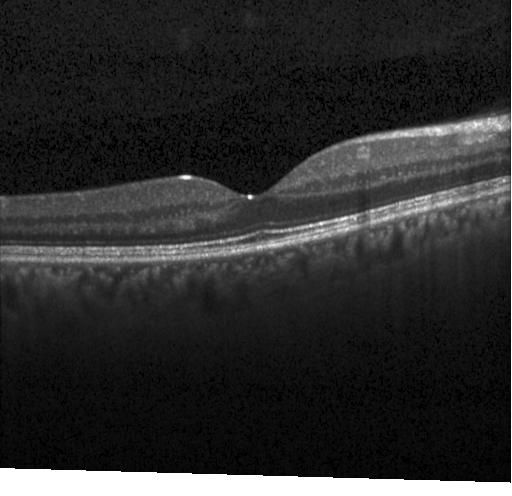

No evidence of choroidal neovascularization, diabetic macular edema, or drusen.